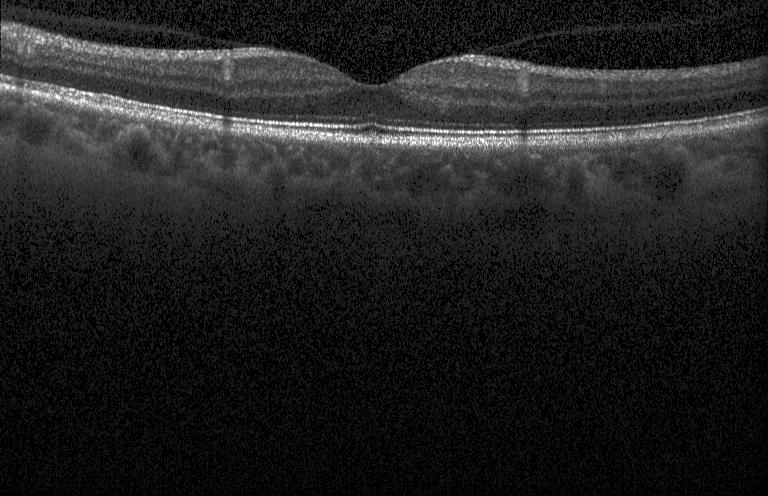 Spectral-domain OCT. Retinal OCT cross-section. Instrument: Heidelberg Spectralis — The scan shows no CNV, DME, or drusen.